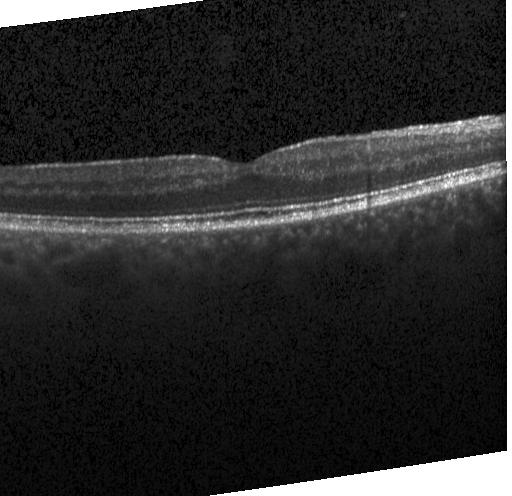
Diagnosis: no evidence of CNV, DME, or drusen.